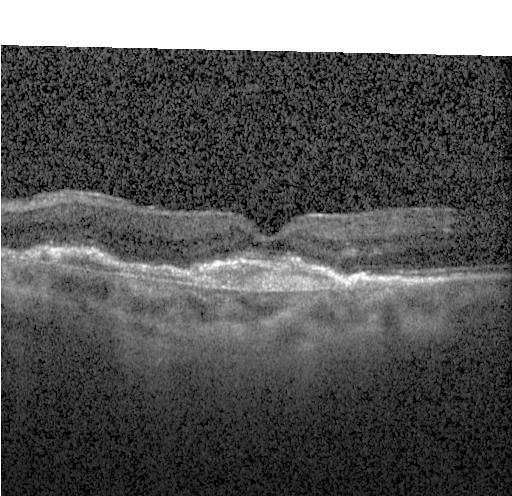

Centered on the fovea, SD-OCT, instrument: Heidelberg Spectralis, optical coherence tomography scan
Diagnosis: CNV.